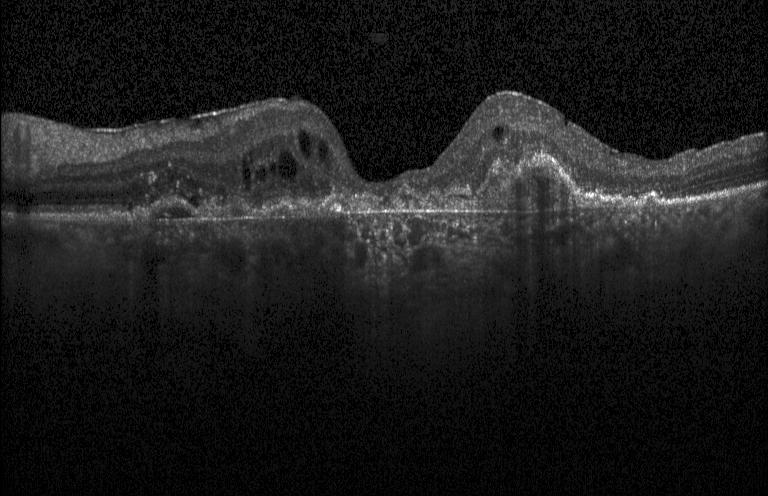
This B-scan demonstrates choroidal neovascularization (CNV).